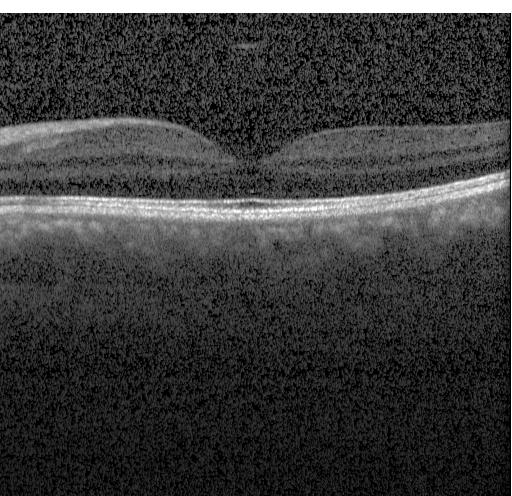
Impression: no CNV, DME, or drusen.